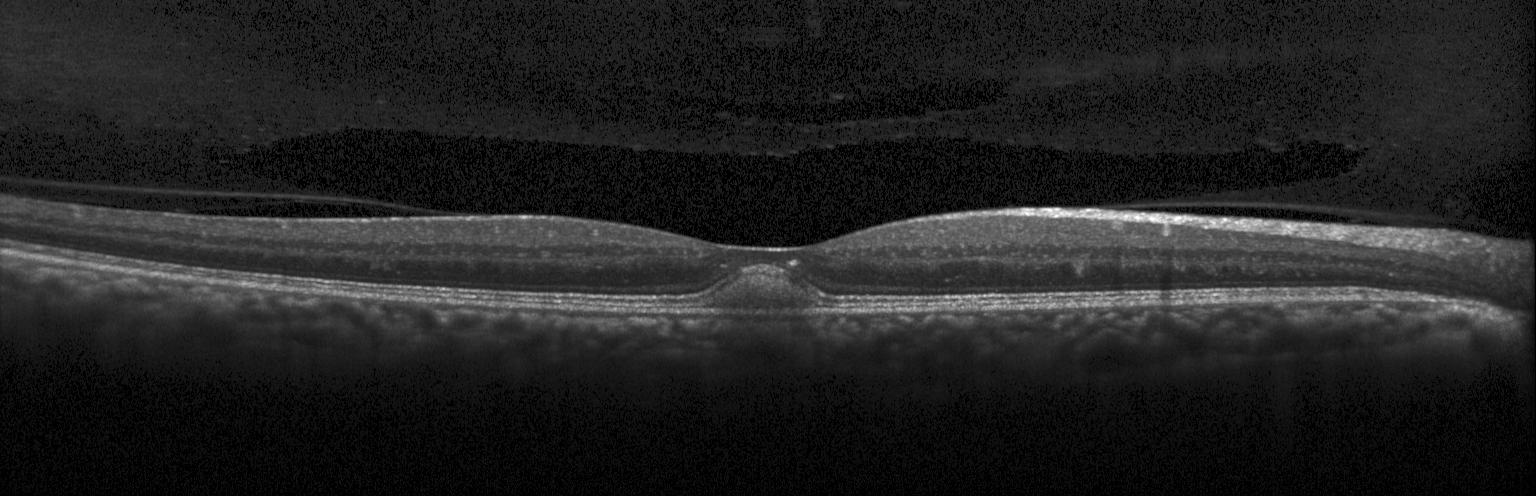

SD-OCT; retinal OCT B-scan; centered on the fovea.
Finding: CNV.